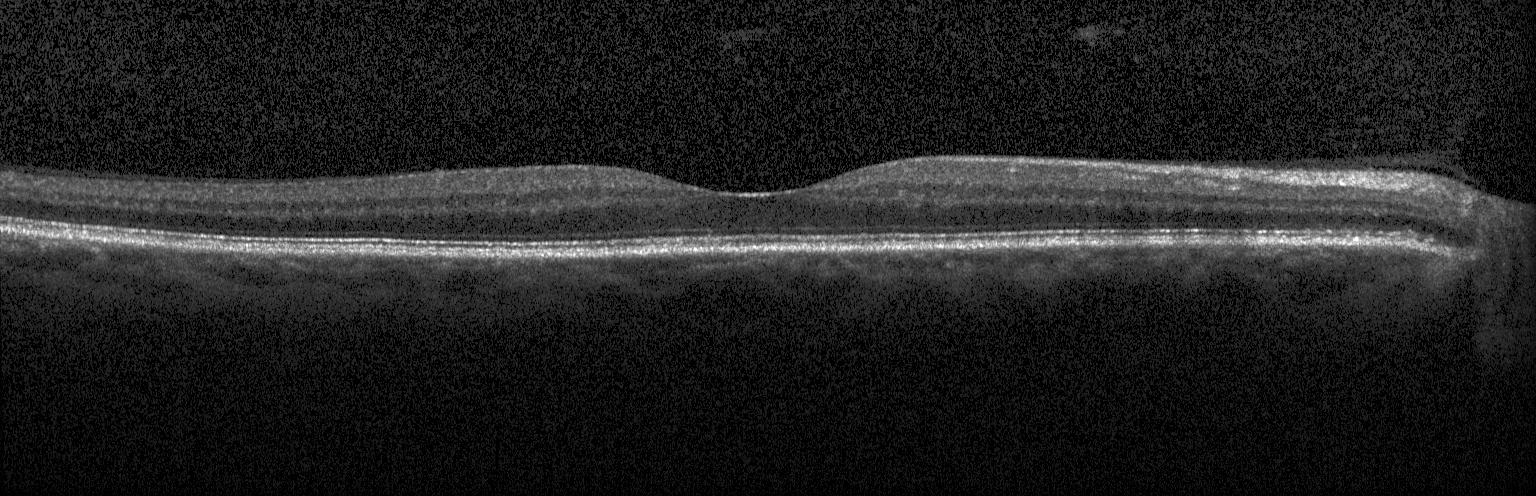

Spectral-domain optical coherence tomography. Optical coherence tomography scan — Diagnosis: no choroidal neovascularization, no diabetic macular edema, and no drusen.